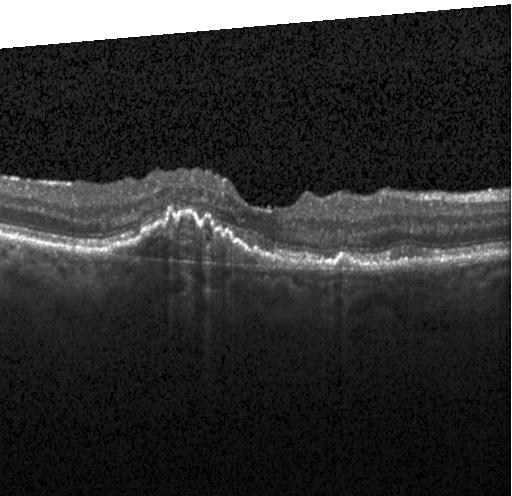 Spectral-domain OCT · retinal OCT B-scan — Finding: CNV.